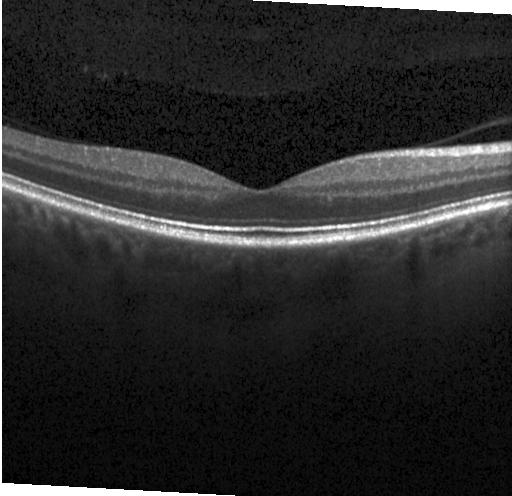
Retinal OCT cross-section showing no CNV, DME, or drusen.